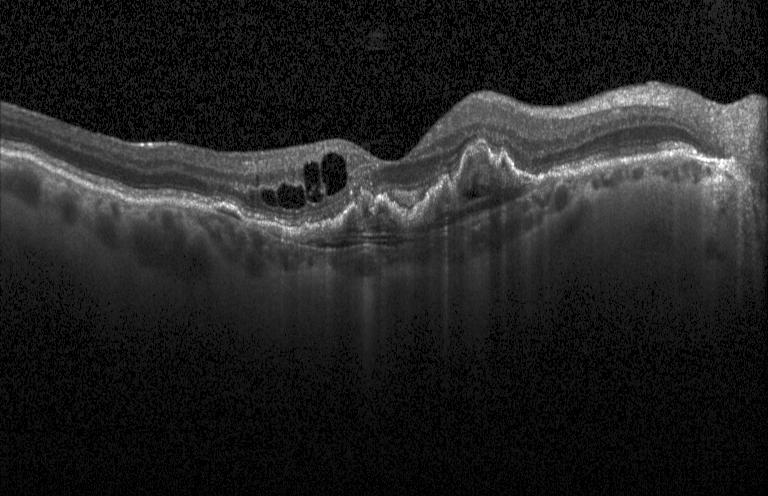 Optical coherence tomography B-scan. A choroidal neovascular membrane.